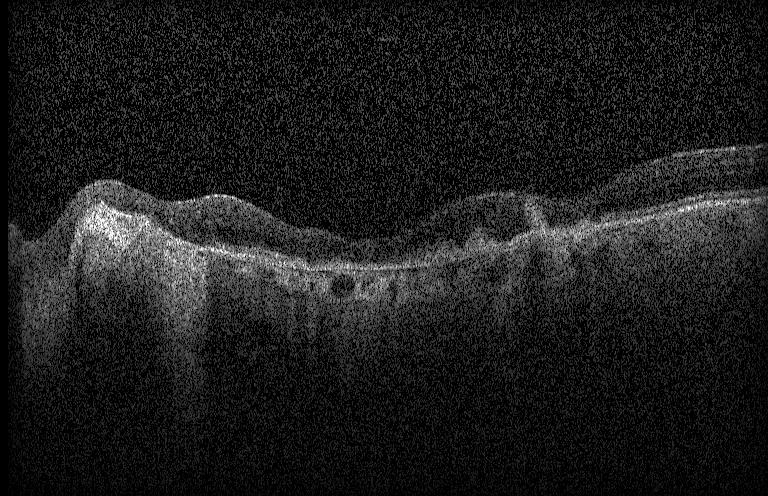
SD-OCT · optical coherence tomography B-scan · Heidelberg Spectralis · through the macula. This B-scan demonstrates a choroidal neovascular membrane.